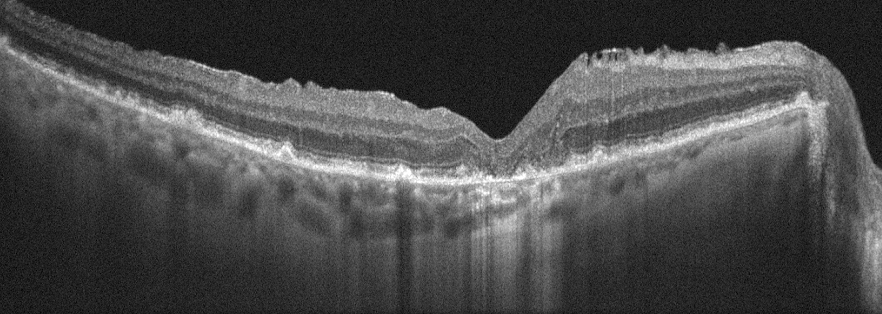
Through the macula. Optical coherence tomography scan. Acquired on an Optovue Avanti RTVue XR. Right eye.
Age-related macular degeneration.